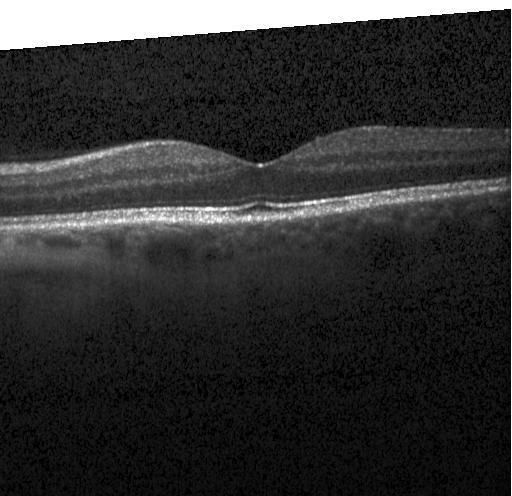

Macular OCT: no evidence of CNV, DME, or drusen.